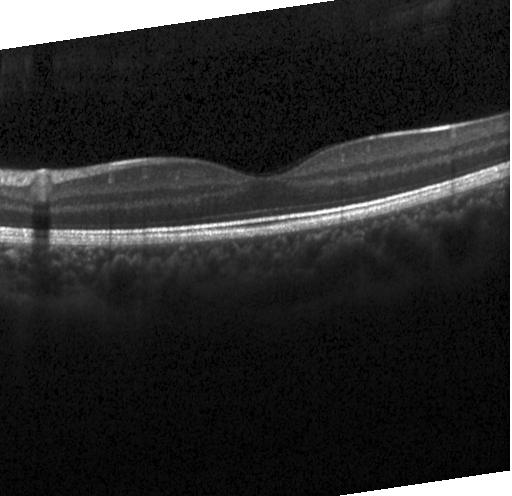 Spectral-domain OCT B-scan: no choroidal neovascularization, diabetic macular edema, or drusen.